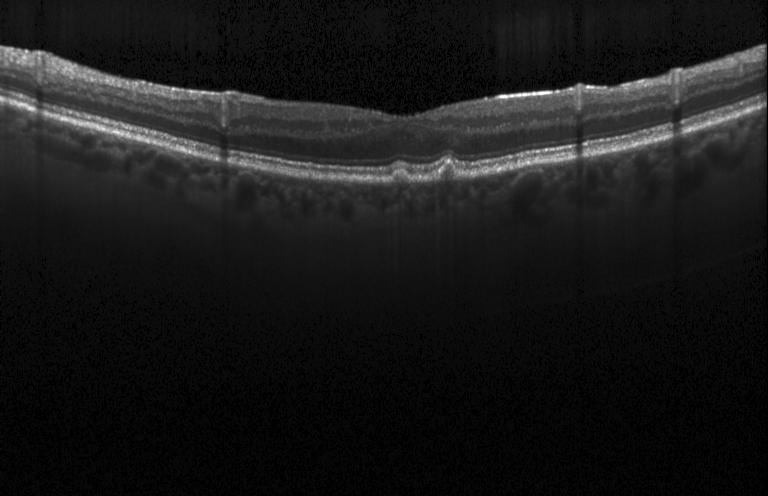
Spectral-domain OCT. Retinal OCT B-scan — The scan shows sub-RPE drusenoid deposits.